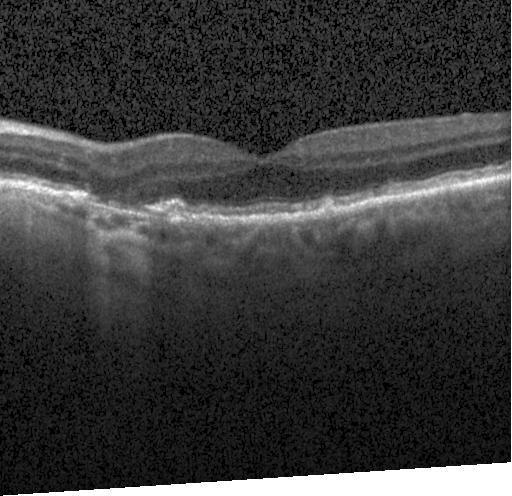 Impression: multiple drusen.